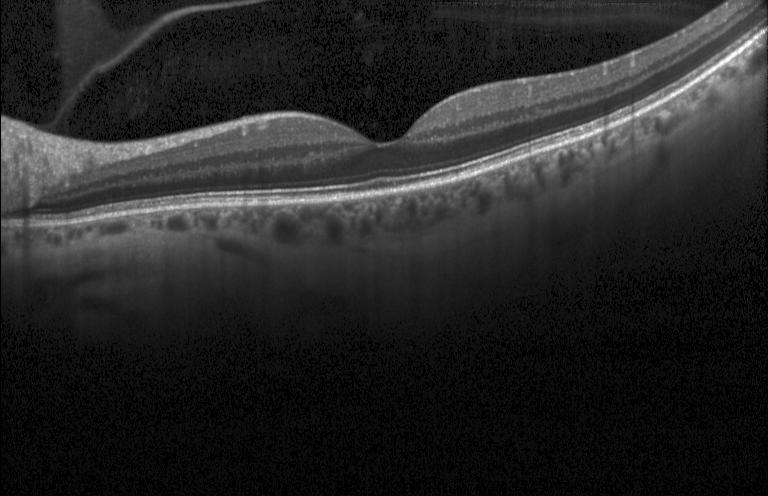

OCT line scan · fovea-centered · spectral-domain optical coherence tomography · Heidelberg Spectralis. No CNV, no DME, and no drusen.